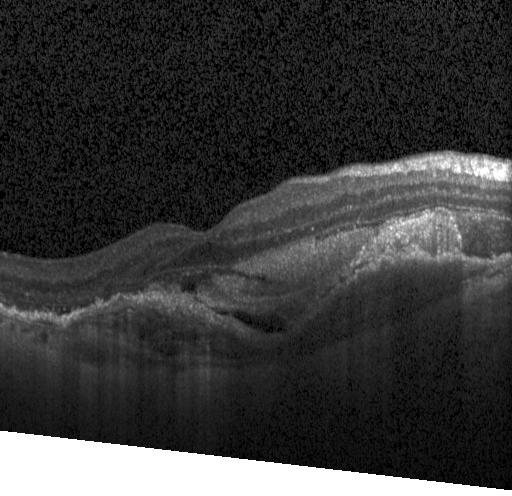
OCT finding: a choroidal neovascular membrane.